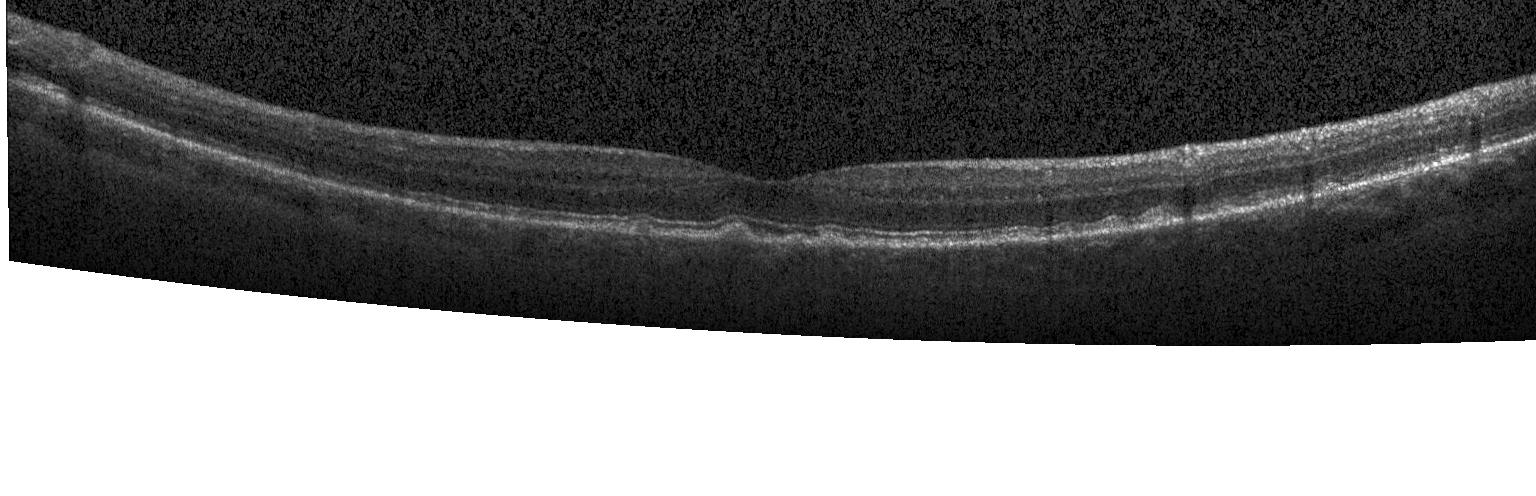 Spectral-domain optical coherence tomography; OCT B-scan; Heidelberg Spectralis OCT system.
This B-scan demonstrates multiple drusen.